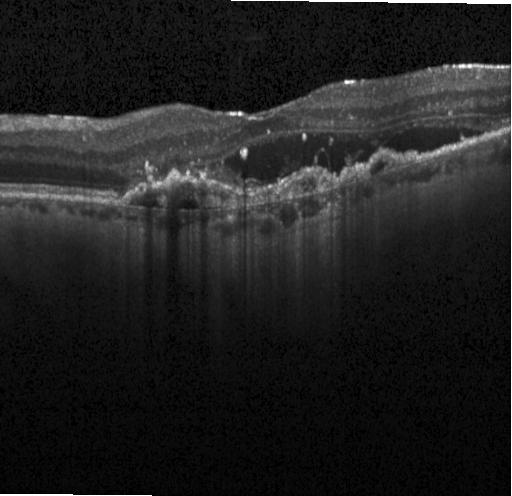 Finding: CNV.